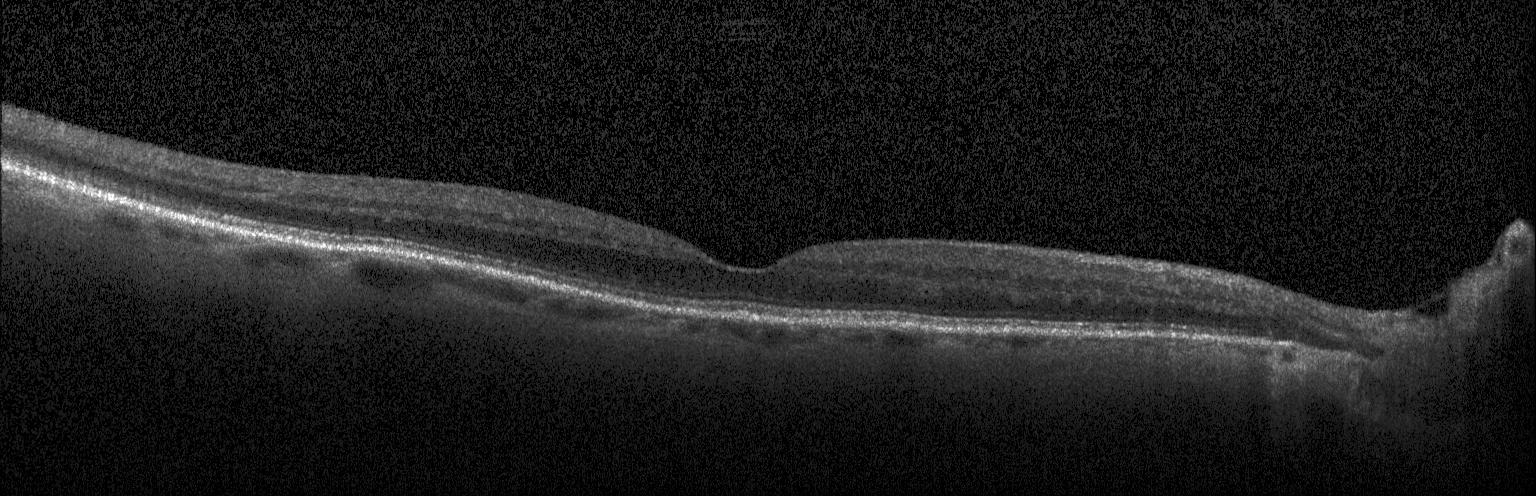
Optical coherence tomography scan
Impression: no CNV, no DME, and no drusen.